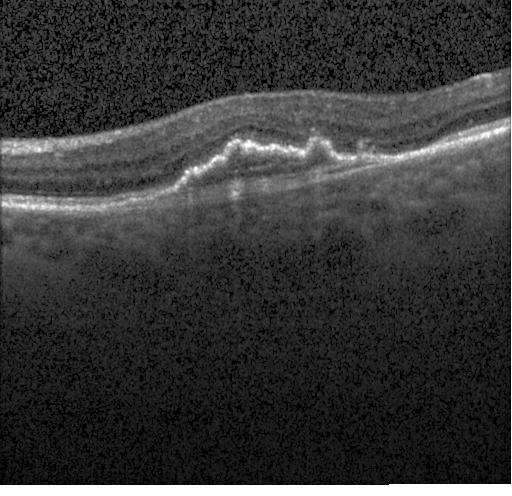
Retinal OCT cross-section, SD-OCT.
This B-scan demonstrates a choroidal neovascular membrane.